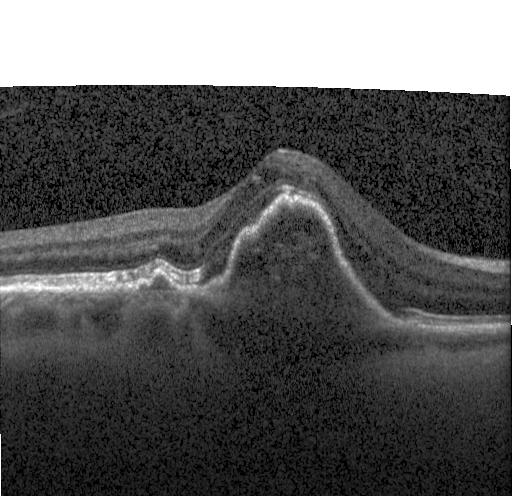
Spectral-domain OCT, retinal OCT B-scan
Impression: choroidal neovascularization.